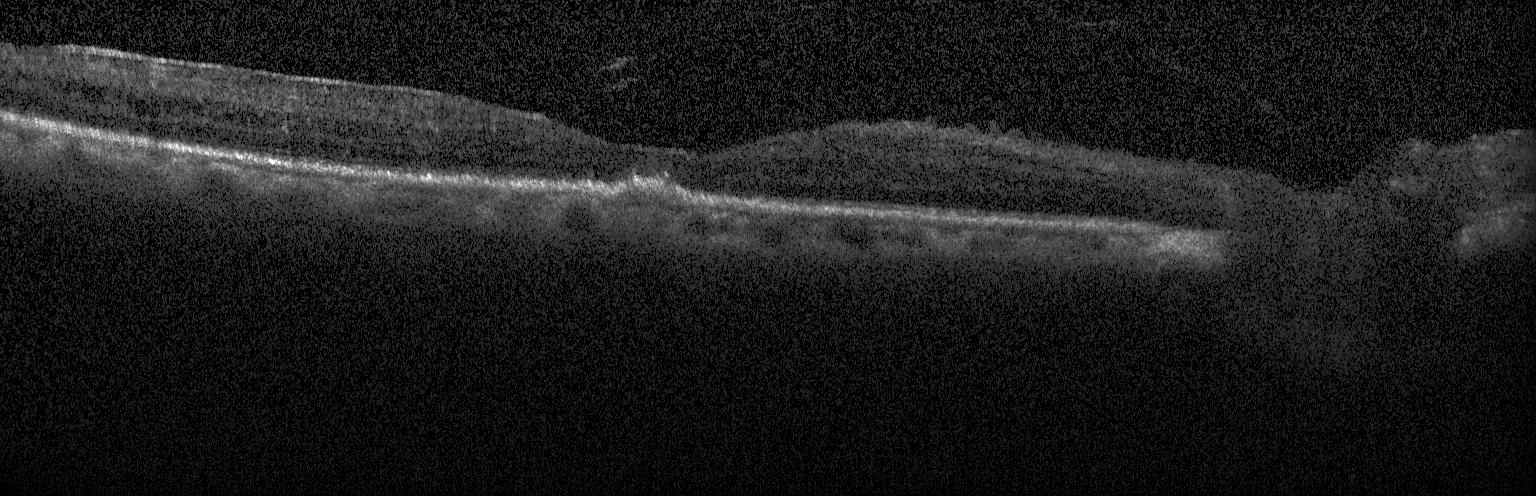
SD-OCT; optical coherence tomography scan
OCT finding: CNV.